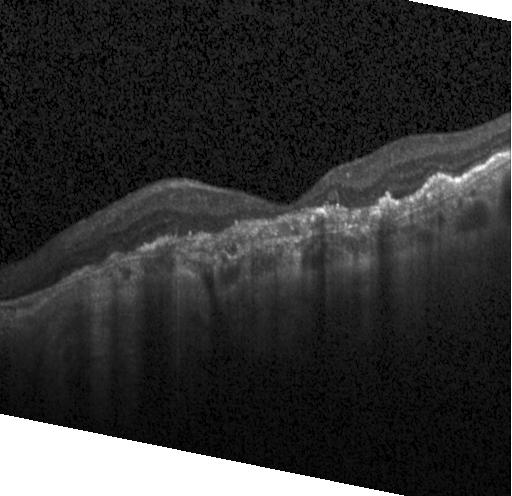 Retinal OCT cross-section showing a choroidal neovascular membrane.